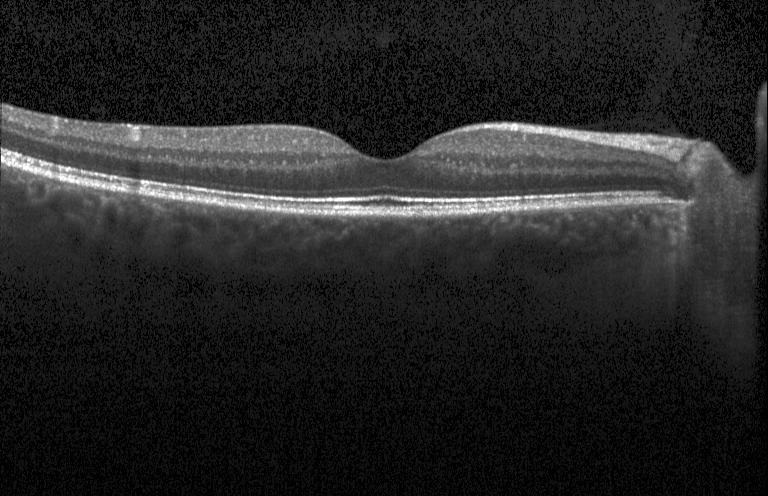

Macular OCT: neither choroidal neovascularization, diabetic macular edema, nor drusen.